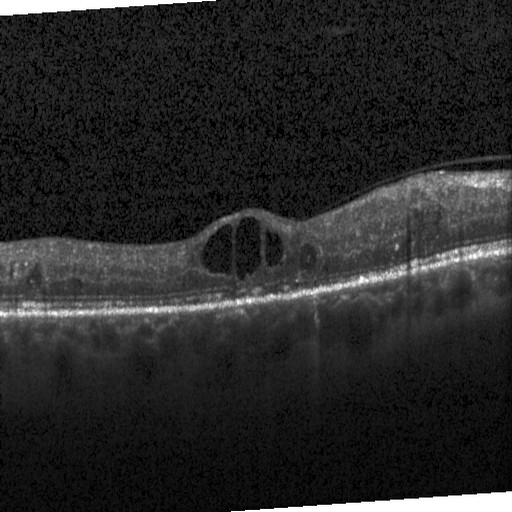

The scan shows diabetic macular edema.